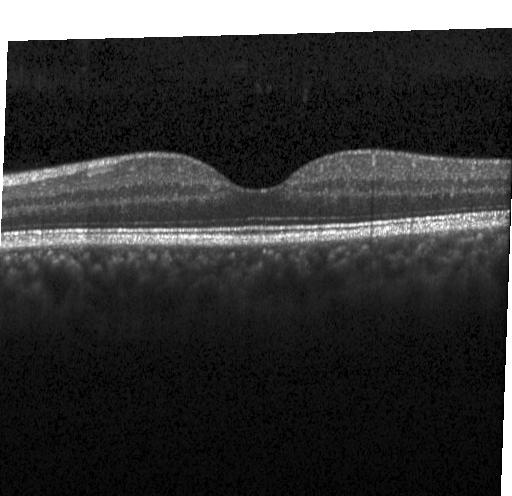
OCT B-scan
Assessment: neither choroidal neovascularization, diabetic macular edema, nor drusen.